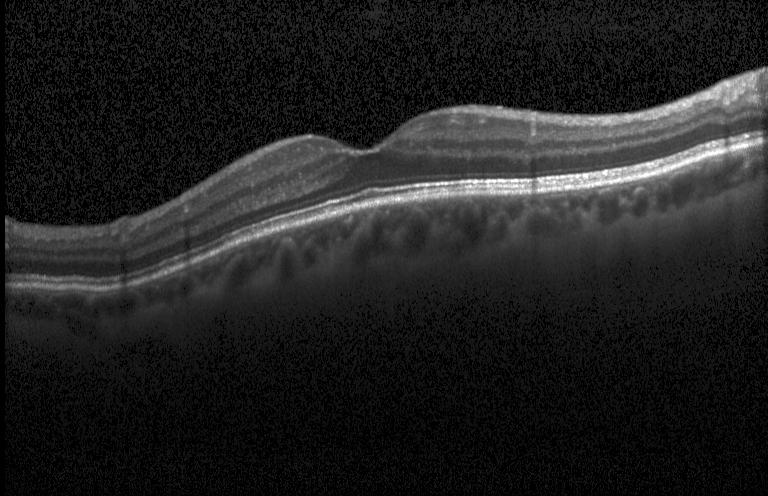

Retinal OCT cross-section
Dx: no choroidal neovascularization, no diabetic macular edema, and no drusen.